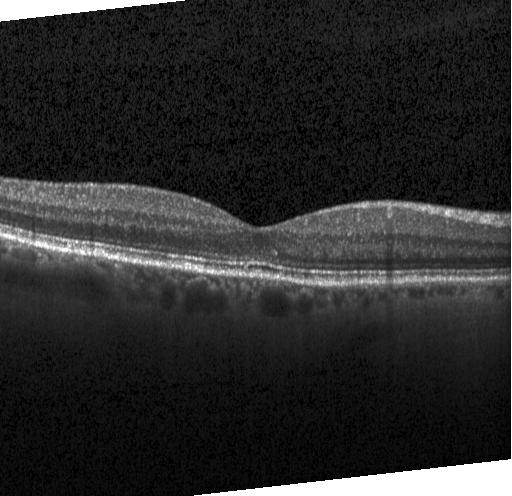
Retinal OCT cross-section showing no CNV, DME, or drusen.